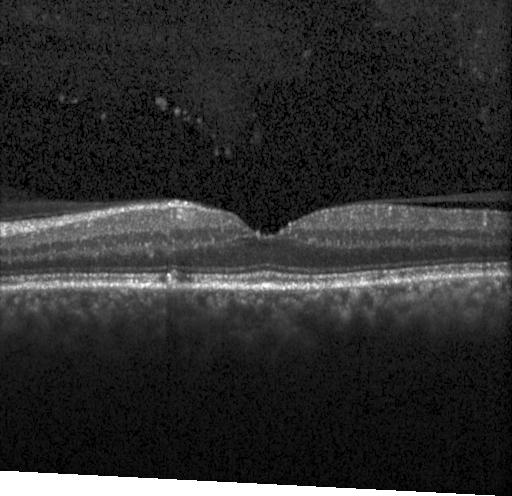

Acquired on a Heidelberg Spectralis; fovea-centered; spectral-domain optical coherence tomography; OCT B-scan.
Dx: multiple drusen.